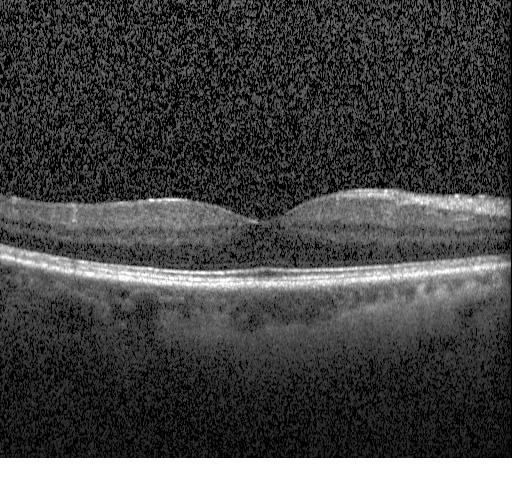
Optical coherence tomography B-scan. Spectral-domain OCT
OCT finding: no choroidal neovascularization, no diabetic macular edema, and no drusen.